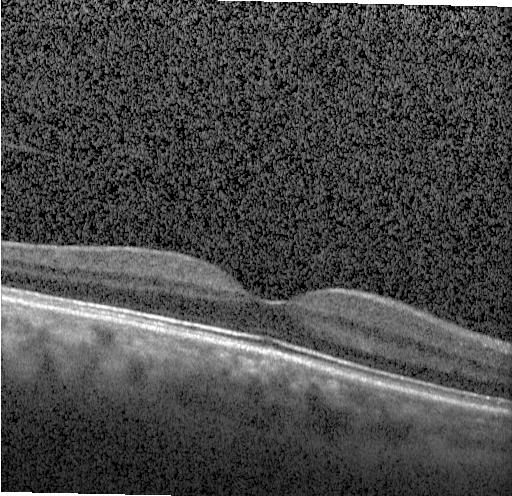

SD-OCT; Heidelberg Spectralis OCT system; retinal OCT cross-section
Macular OCT: no choroidal neovascularization, diabetic macular edema, or drusen.